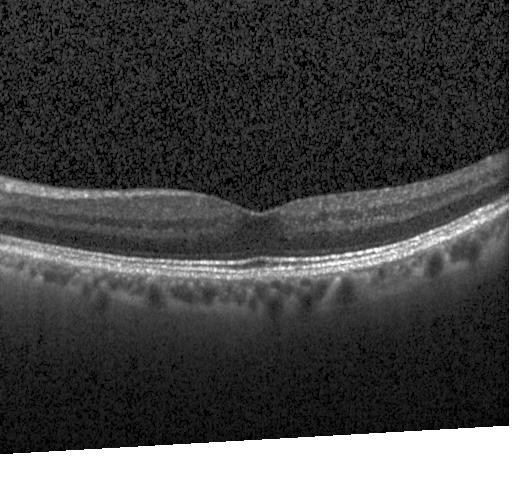
OCT finding: neither choroidal neovascularization, diabetic macular edema, nor drusen.